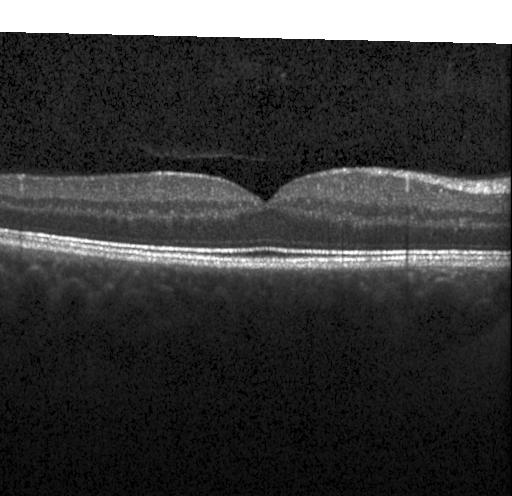
Optical coherence tomography B-scan.
This B-scan demonstrates neither choroidal neovascularization, diabetic macular edema, nor drusen.